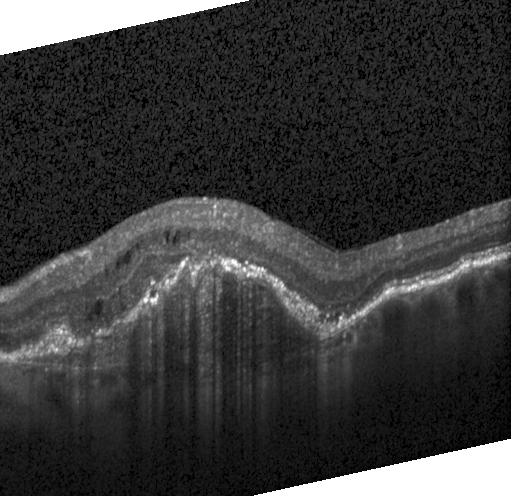

Heidelberg Spectralis; horizontal scan through the fovea; SD-OCT; optical coherence tomography B-scan — Finding: CNV.